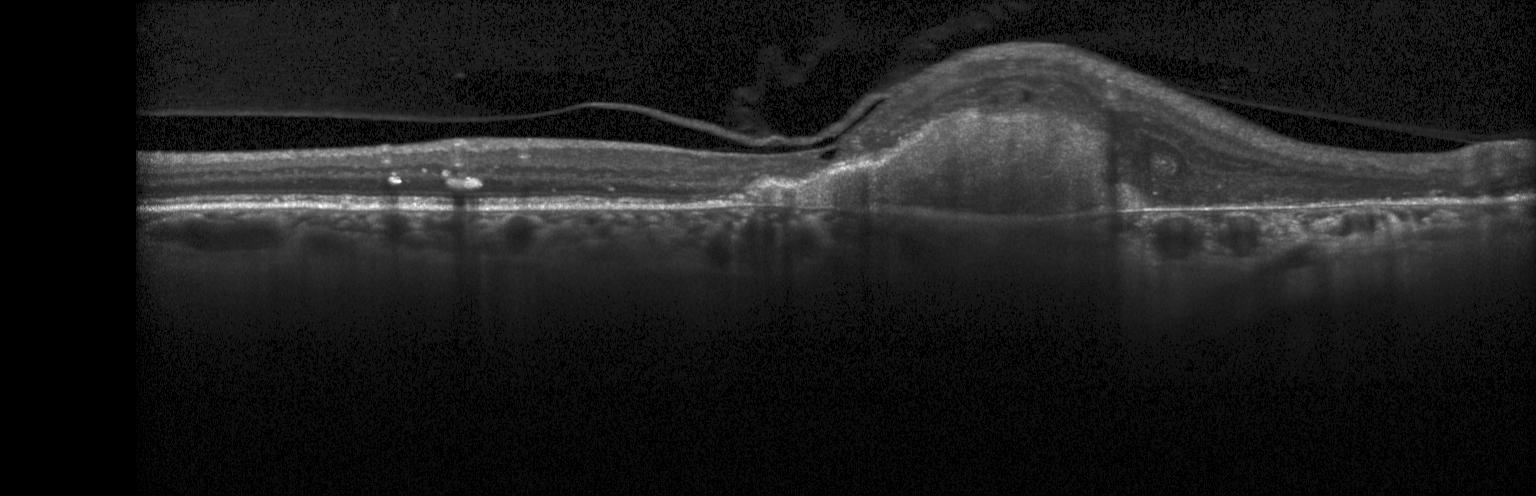
Centered on the fovea; OCT line scan — A choroidal neovascular membrane.